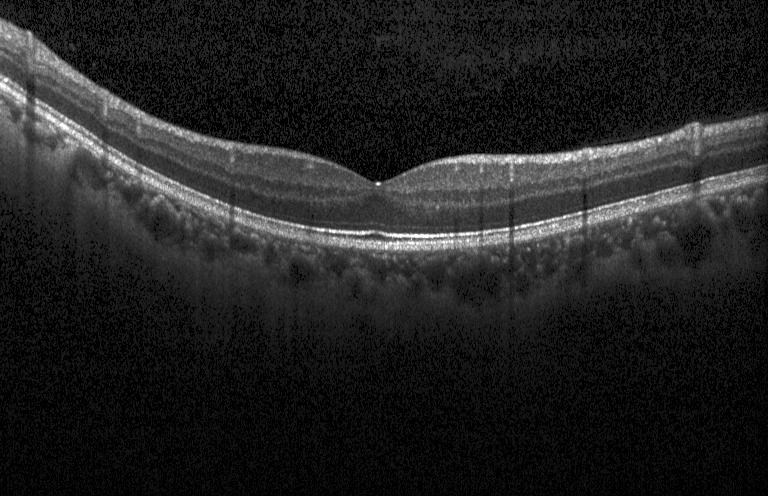

Spectral-domain OCT B-scan: no evidence of choroidal neovascularization, diabetic macular edema, or drusen.